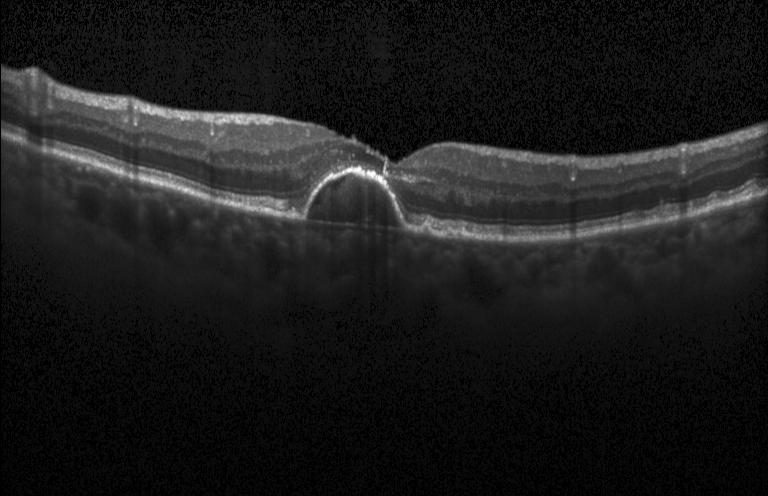

The scan shows a choroidal neovascular membrane.